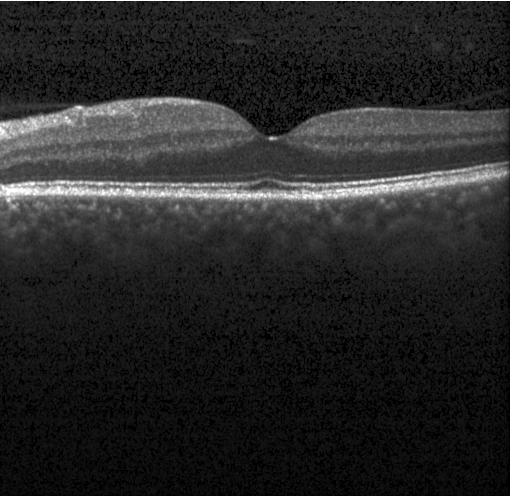

SD-OCT; acquired on a Heidelberg Spectralis; OCT B-scan; macular scan
This B-scan demonstrates no evidence of choroidal neovascularization, diabetic macular edema, or drusen.